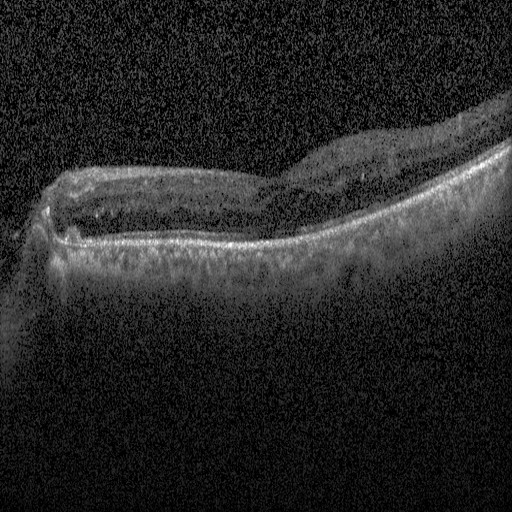
Retinal OCT cross-section showing diabetic macular edema (DME).